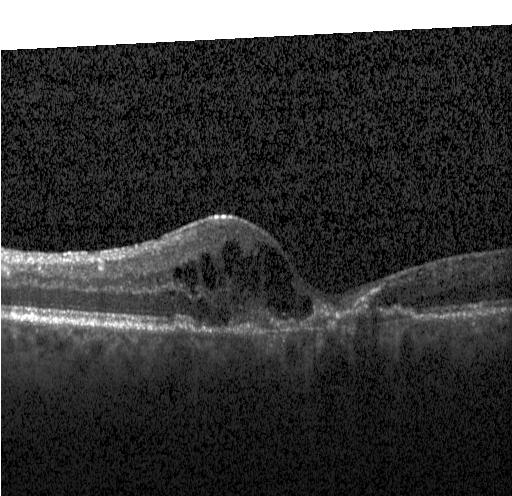

Spectral-domain optical coherence tomography. Retinal OCT cross-section — Impression: a choroidal neovascular membrane.